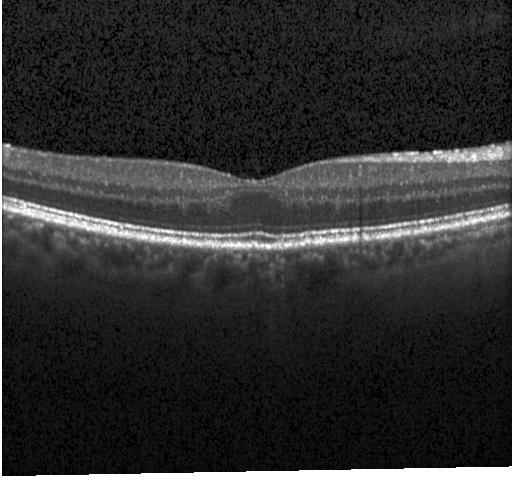
Acquired on a Heidelberg Spectralis, retinal OCT cross-section, through the macula, spectral-domain OCT.
Dx: no CNV, DME, or drusen.